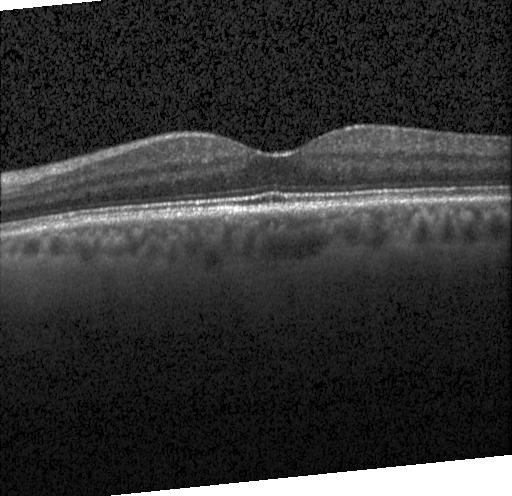 SD-OCT · centered on the fovea · retinal OCT B-scan — OCT finding: no choroidal neovascularization, diabetic macular edema, or drusen.